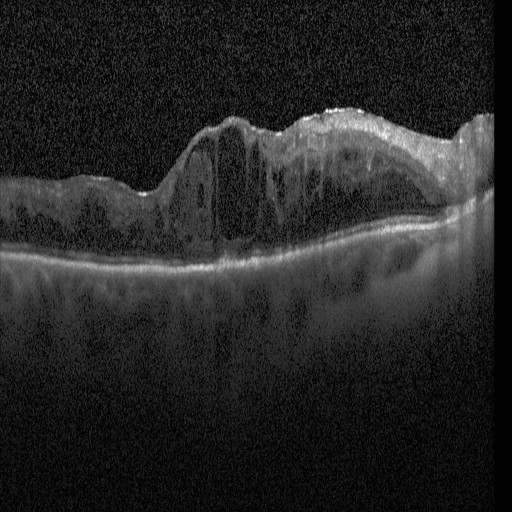
Finding: diabetic macular edema.